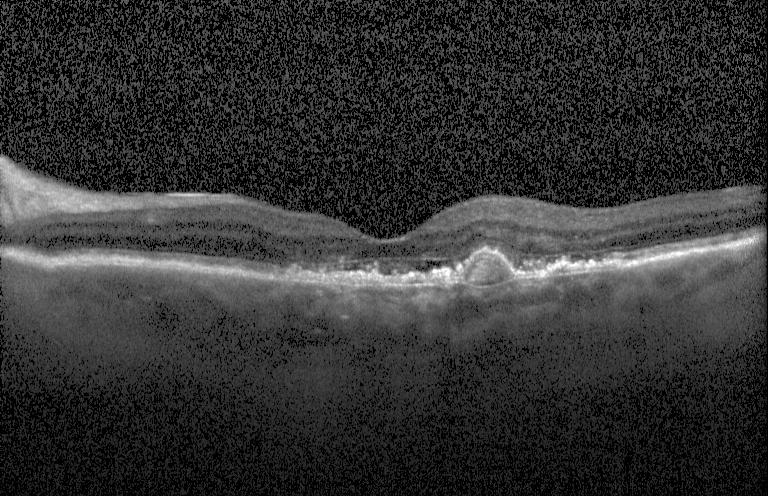

SD-OCT, Heidelberg Spectralis, OCT line scan — Finding: a choroidal neovascular membrane.